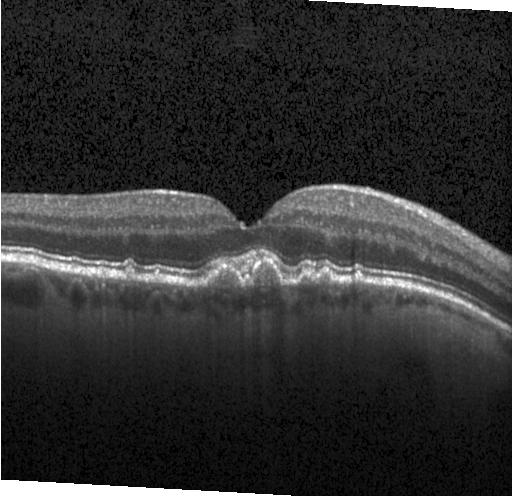

Instrument: Heidelberg Spectralis, spectral-domain optical coherence tomography, retinal OCT cross-section, horizontal scan through the fovea. Diagnosis: multiple drusen.